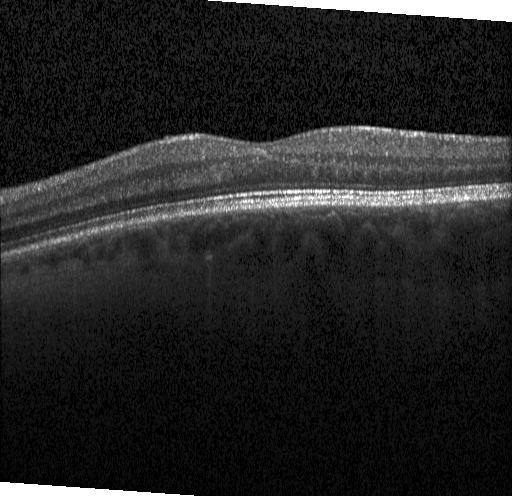 Diagnosis: no CNV, DME, or drusen.